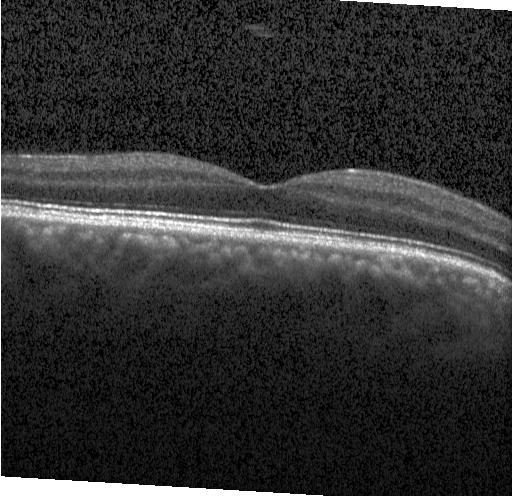 Assessment: no CNV, no DME, and no drusen.